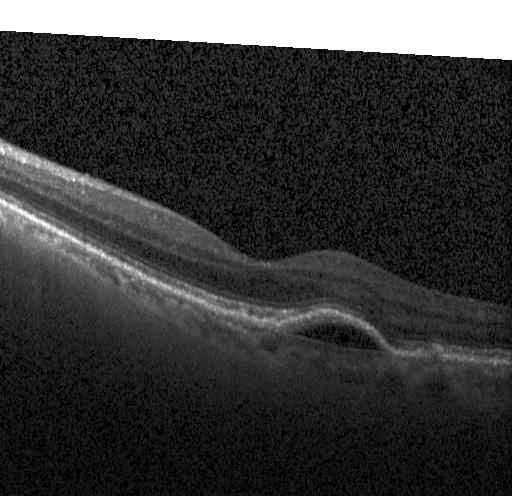 Spectral-domain OCT B-scan: CNV.